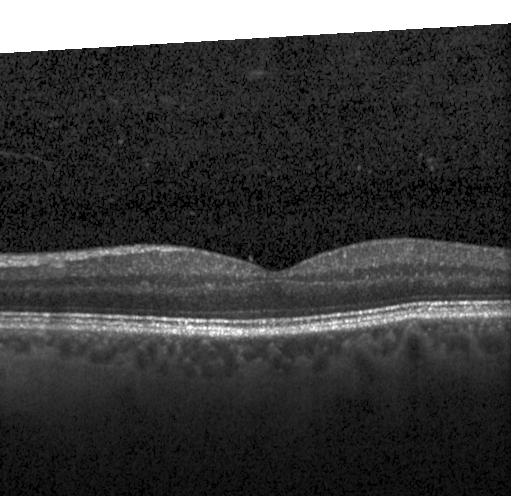 OCT scan showing no evidence of choroidal neovascularization, diabetic macular edema, or drusen.